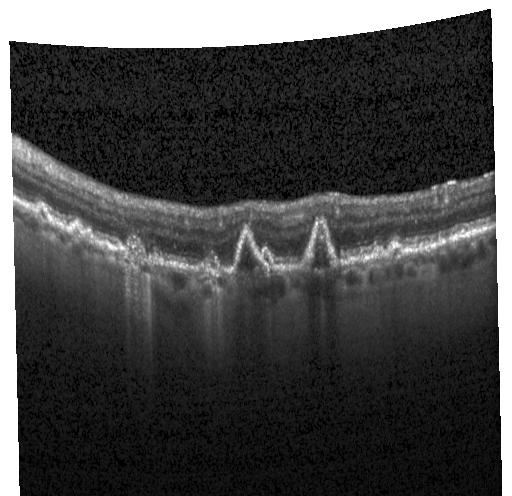 Macular scan; Heidelberg Spectralis OCT system; SD-OCT; optical coherence tomography scan. Diagnosis: choroidal neovascularization.